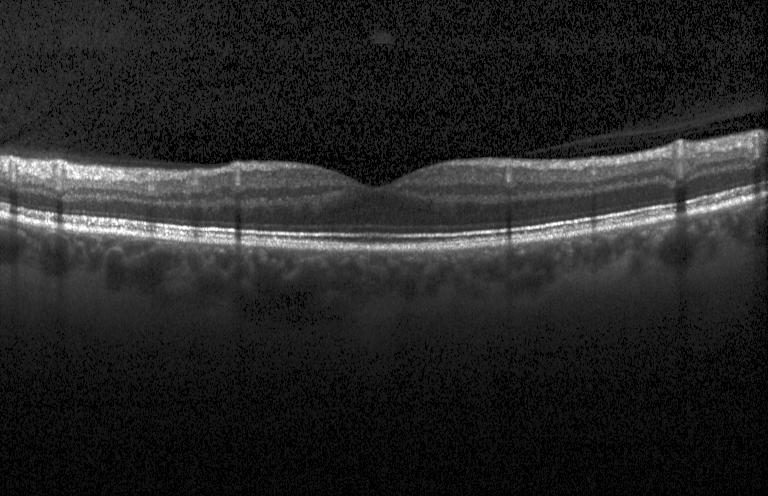 Optical coherence tomography B-scan · spectral-domain OCT.
Impression: neither CNV, DME, nor drusen.